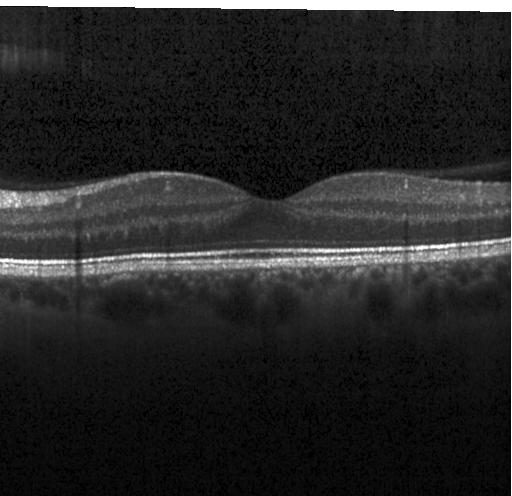
OCT line scan, instrument: Heidelberg Spectralis, fovea-centered
Macular OCT: no CNV, no DME, and no drusen.